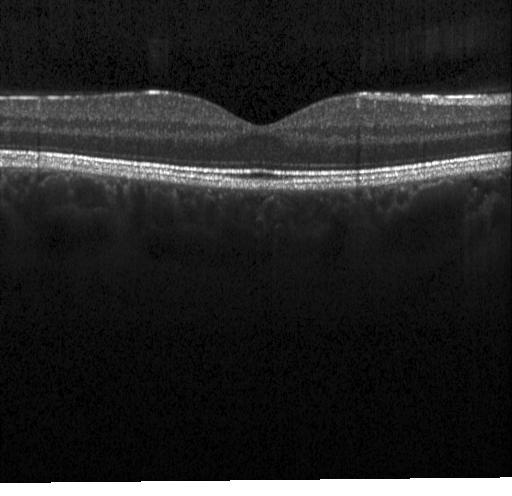
Retinal OCT cross-section showing neither choroidal neovascularization, diabetic macular edema, nor drusen.